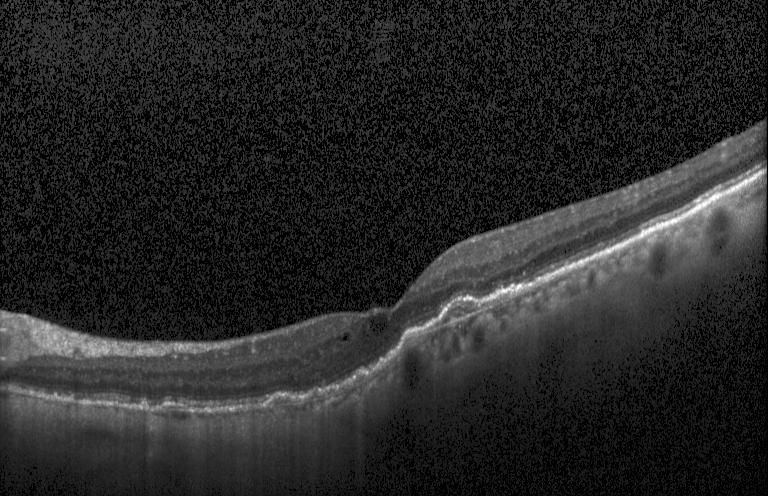
Diagnosis: choroidal neovascularization.